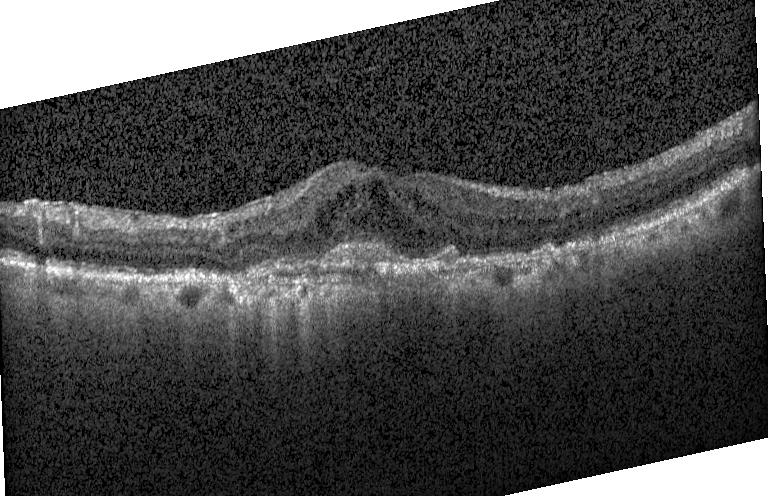
Optical coherence tomography scan, horizontal scan through the fovea, acquired on a Heidelberg Spectralis.
Macular OCT: a choroidal neovascular membrane.